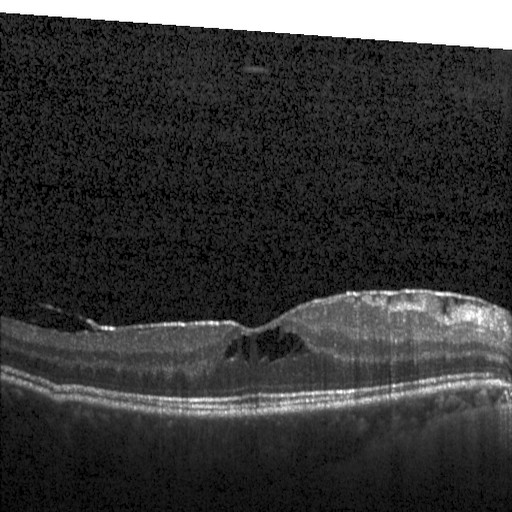

Macular OCT: diabetic macular edema.